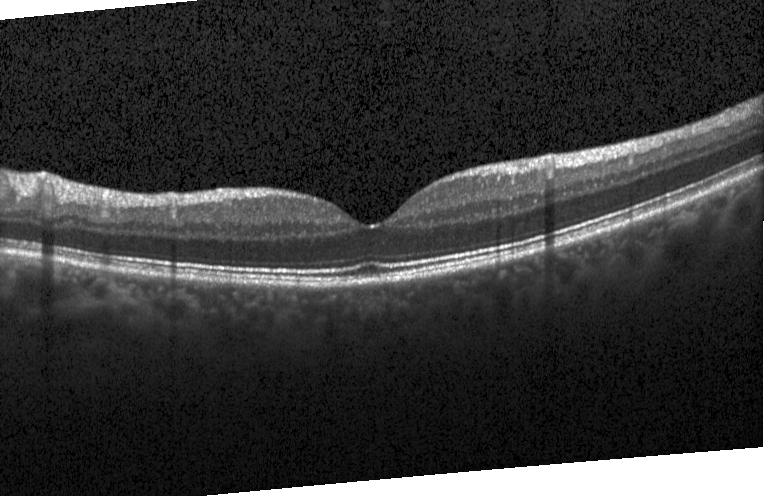
Heidelberg Spectralis OCT system. SD-OCT. Macular scan. Optical coherence tomography scan
No choroidal neovascularization, diabetic macular edema, or drusen.